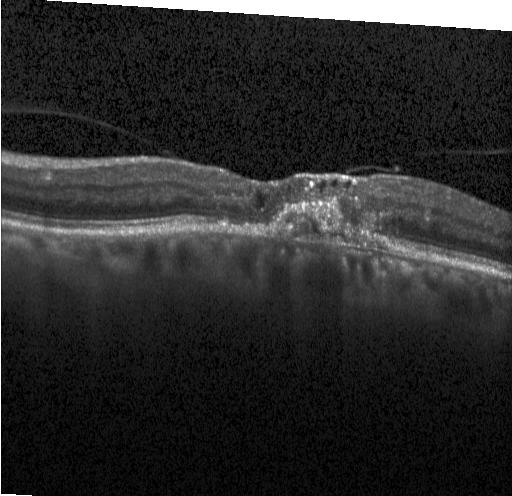
Spectral-domain optical coherence tomography. Optical coherence tomography B-scan.
Diagnosis: CNV.